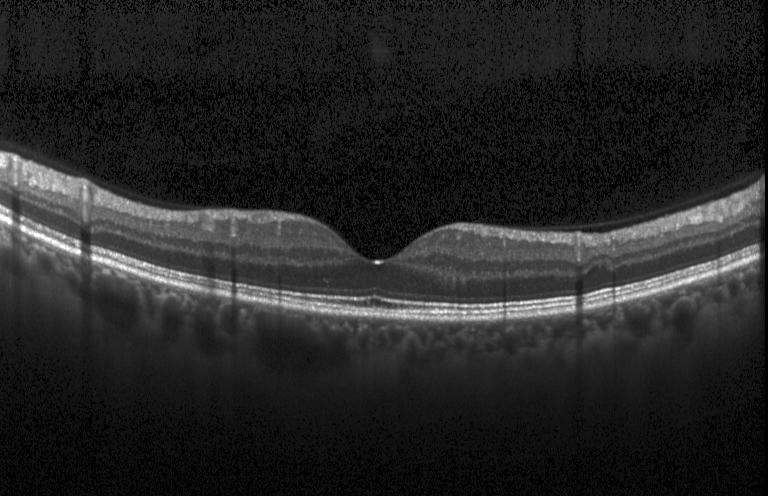 Spectral-domain optical coherence tomography; fovea-centered; instrument: Heidelberg Spectralis; OCT line scan. Diagnosis: no choroidal neovascularization, diabetic macular edema, or drusen.